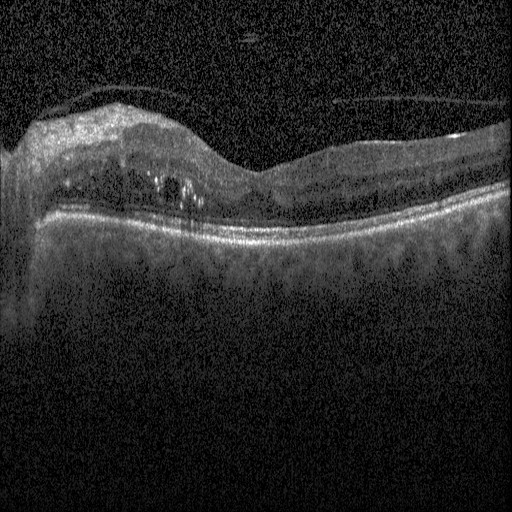 Dx: DME.